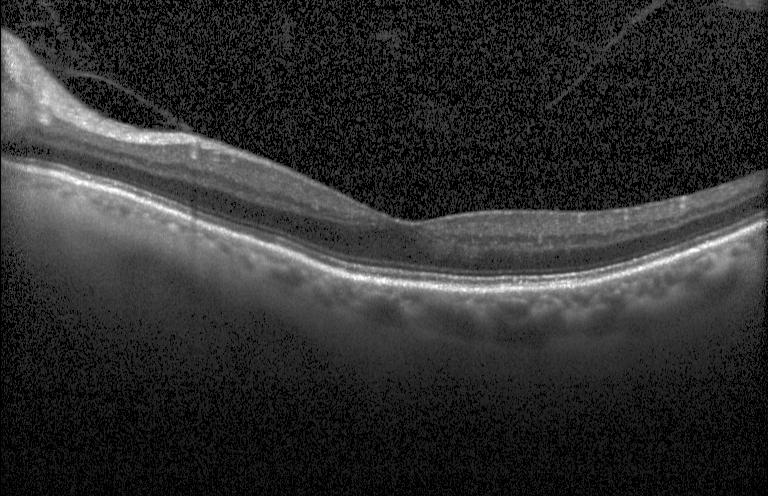

Dx: no evidence of choroidal neovascularization, diabetic macular edema, or drusen.